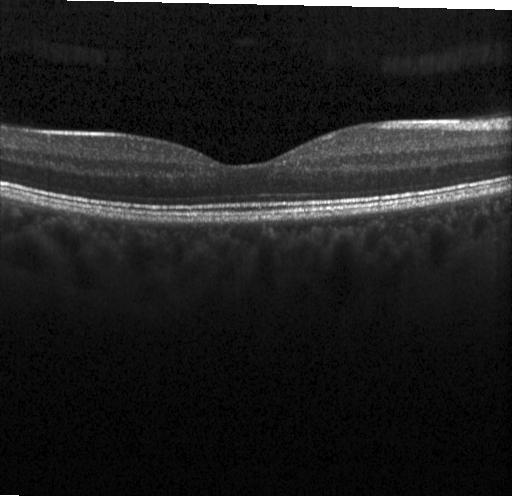

Impression: no choroidal neovascularization, diabetic macular edema, or drusen.